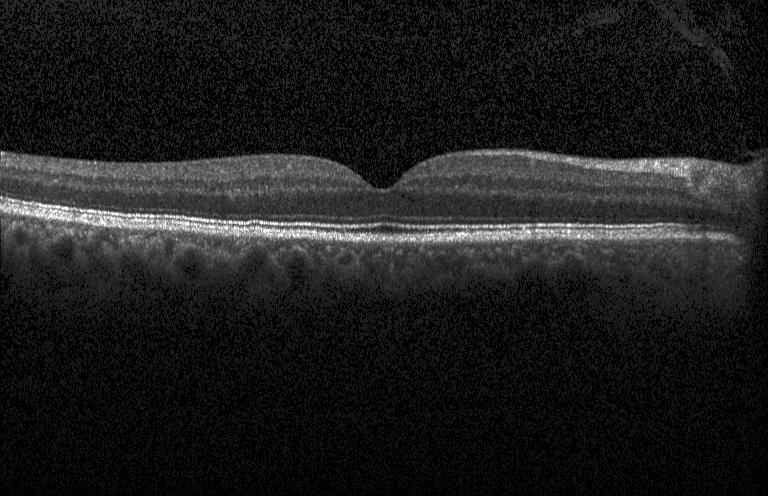 Centered on the fovea · OCT B-scan — Neither choroidal neovascularization, diabetic macular edema, nor drusen.